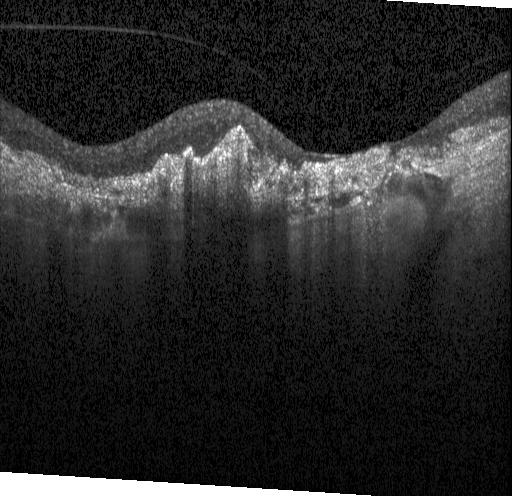
Spectral-domain optical coherence tomography. Acquired on a Heidelberg Spectralis. Optical coherence tomography B-scan — Diagnosis: choroidal neovascularization.